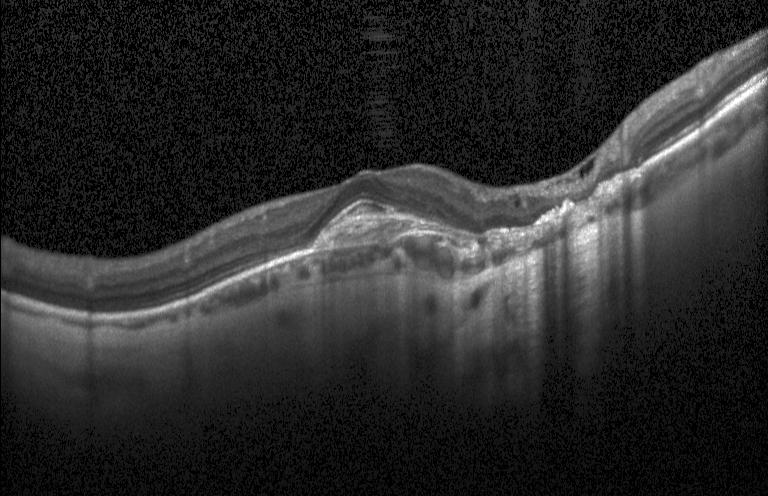 OCT line scan; Heidelberg Spectralis OCT system.
Assessment: a choroidal neovascular membrane.